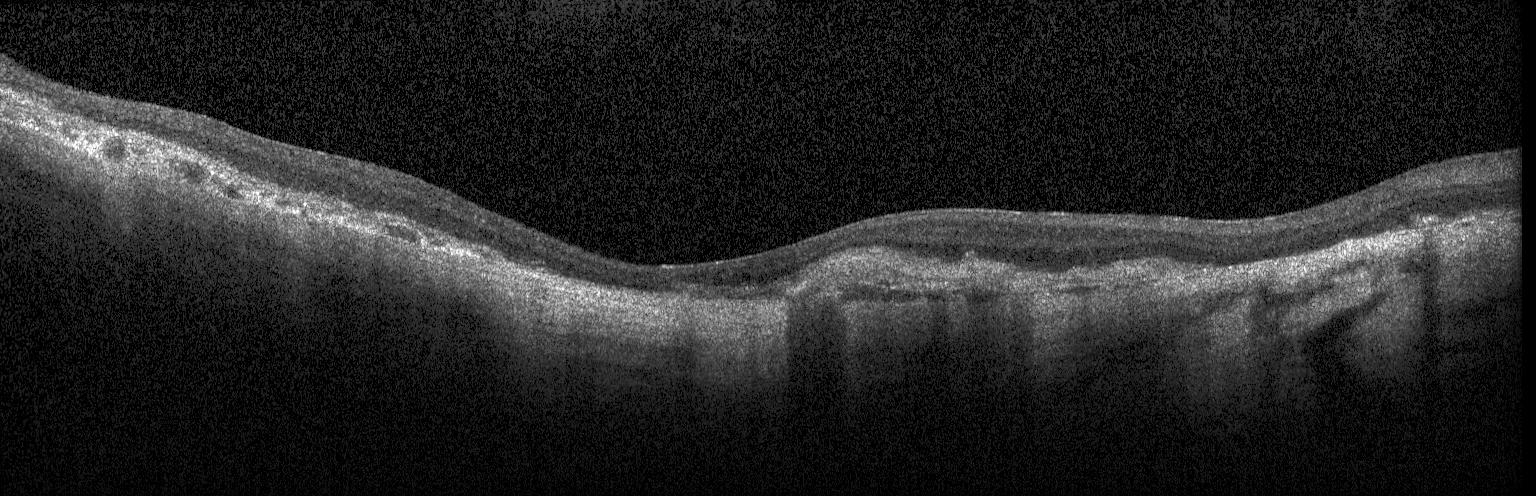

Diagnosis: a choroidal neovascular membrane.